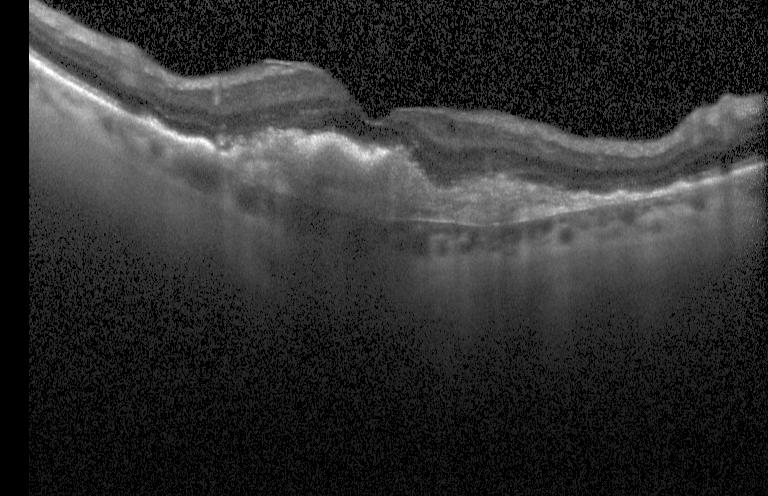

Diagnosis: CNV.